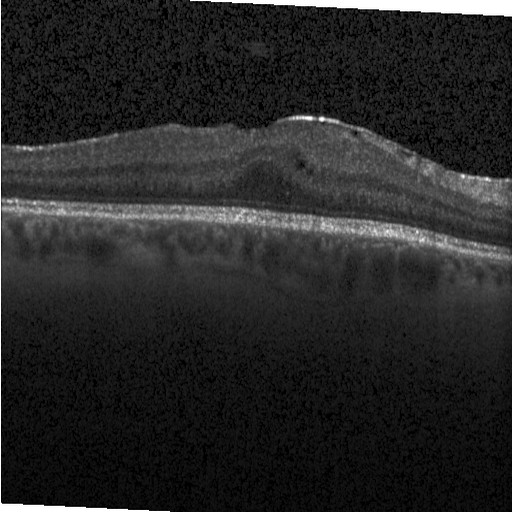

Diagnosis: diabetic macular edema.